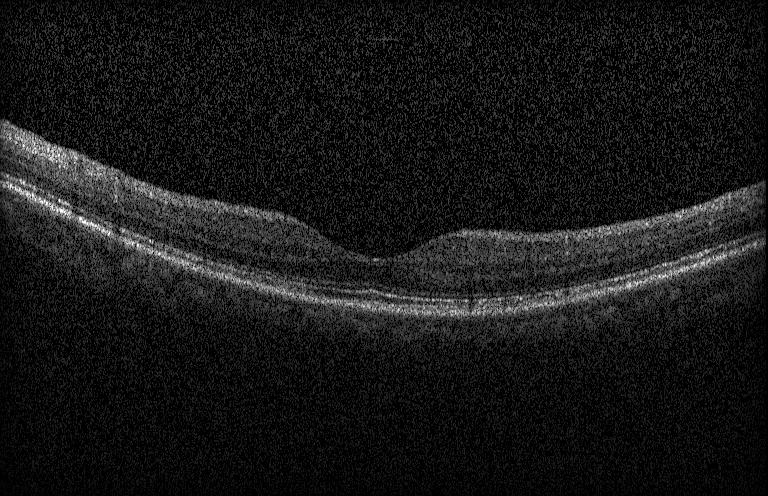

Finding: no CNV, no DME, and no drusen.